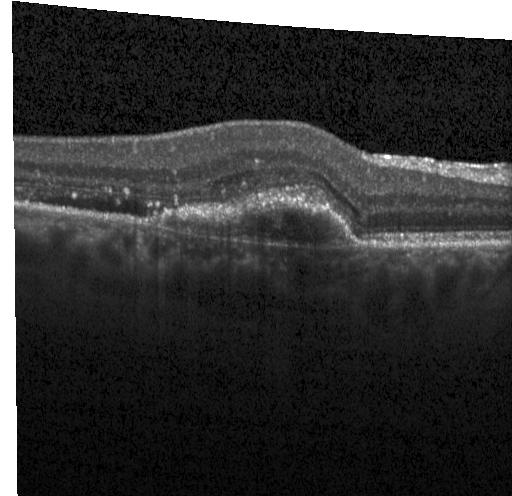
Centered on the fovea, Heidelberg Spectralis, OCT line scan. Dx: choroidal neovascularization.